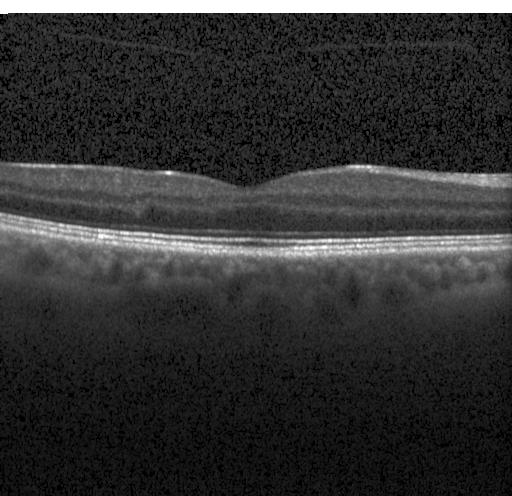
OCT B-scan — The scan shows no CNV, DME, or drusen.